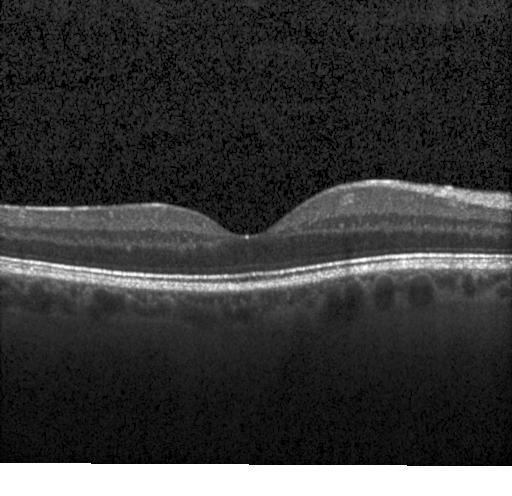
OCT B-scan, spectral-domain OCT
Diagnosis: no choroidal neovascularization, diabetic macular edema, or drusen.